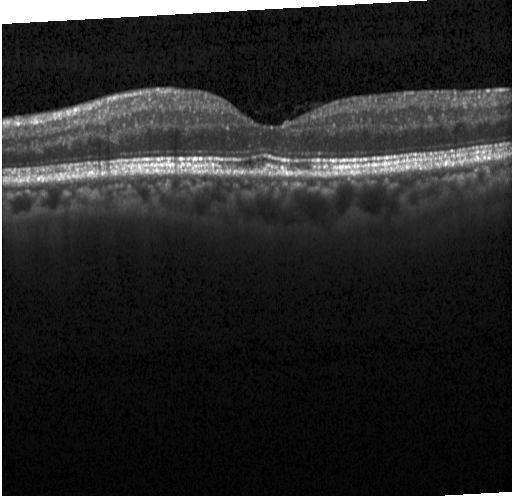 Heidelberg Spectralis OCT system; retinal OCT B-scan
Impression: no evidence of choroidal neovascularization, diabetic macular edema, or drusen.